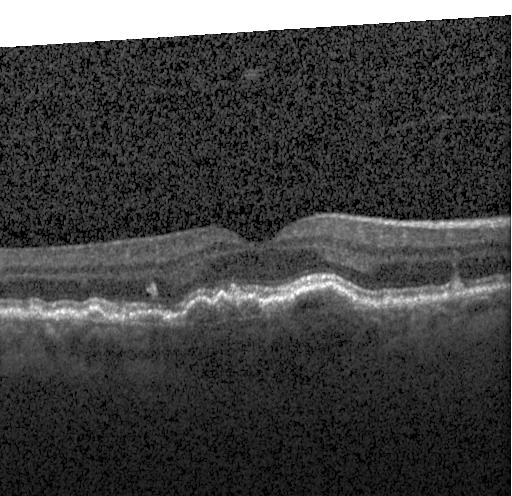
Dx: CNV.